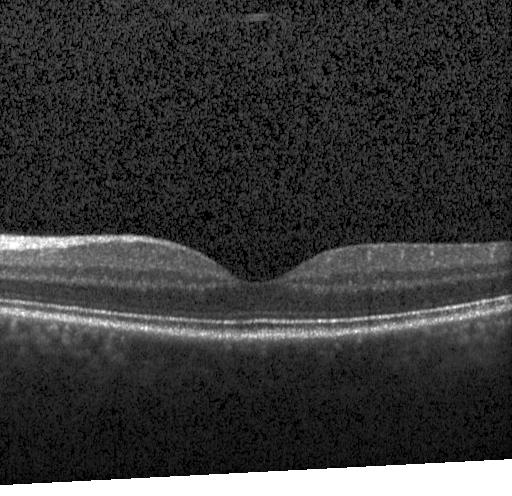 Finding: no choroidal neovascularization, diabetic macular edema, or drusen.